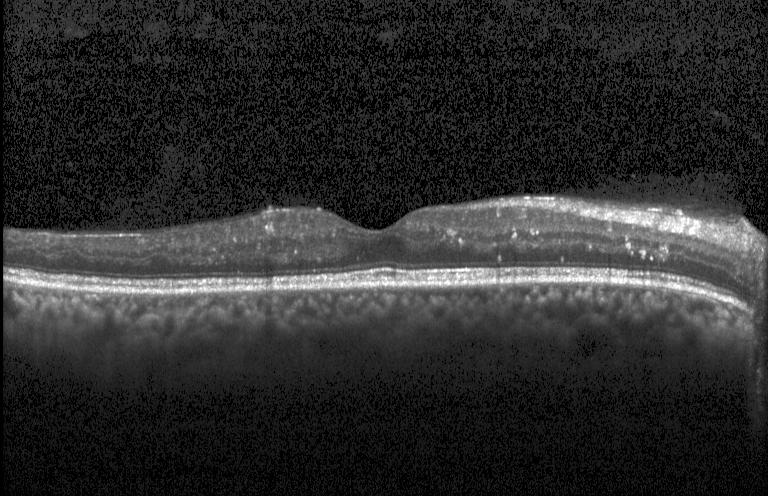
Diagnosis: DME.